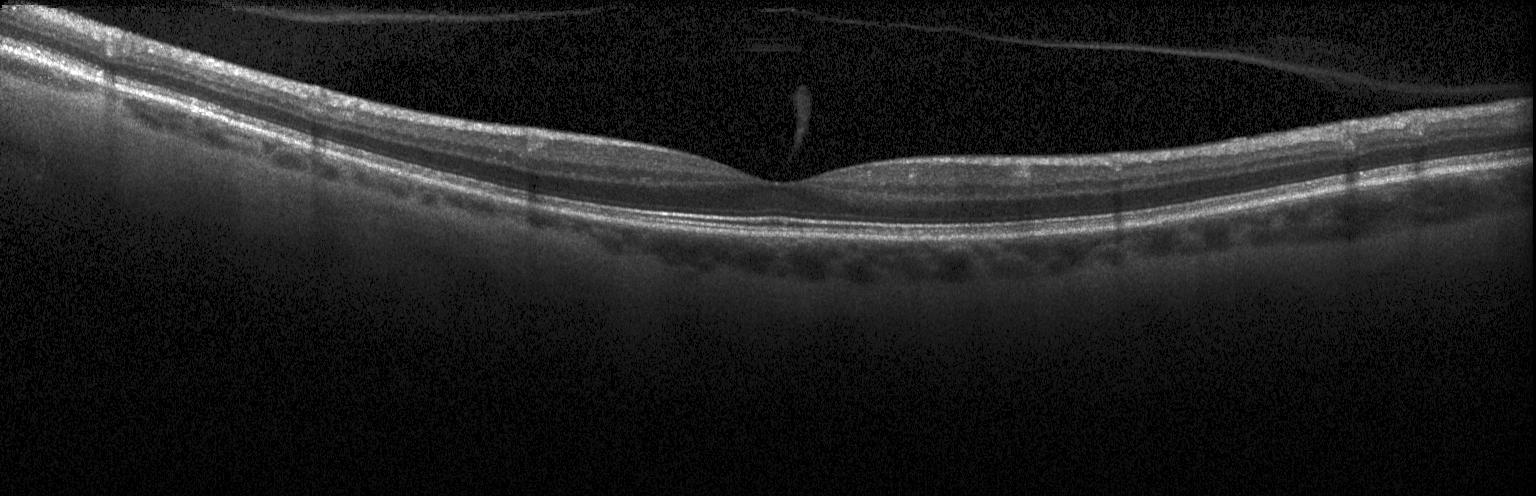 Macular OCT demonstrating no CNV, no DME, and no drusen.